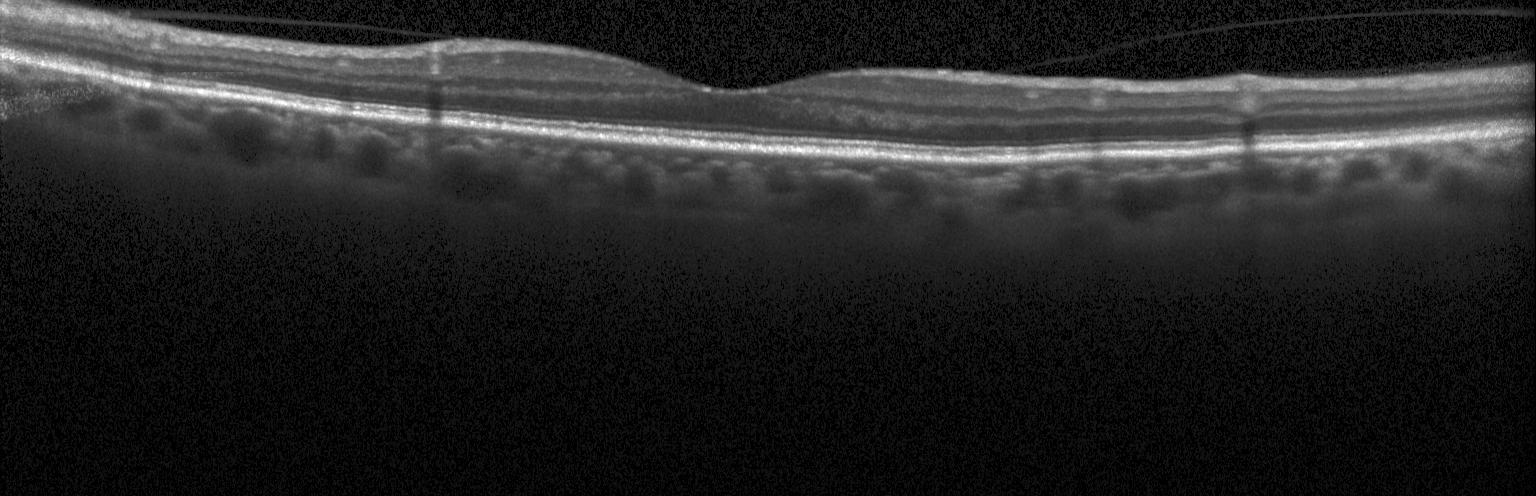
No choroidal neovascularization, diabetic macular edema, or drusen.